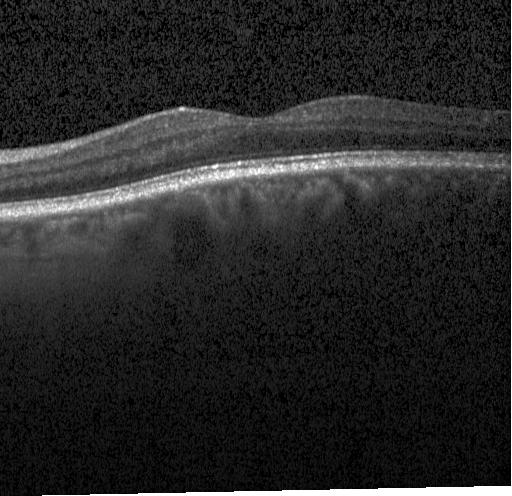

Instrument: Heidelberg Spectralis; centered on the fovea; OCT B-scan — Dx: no evidence of choroidal neovascularization, diabetic macular edema, or drusen.